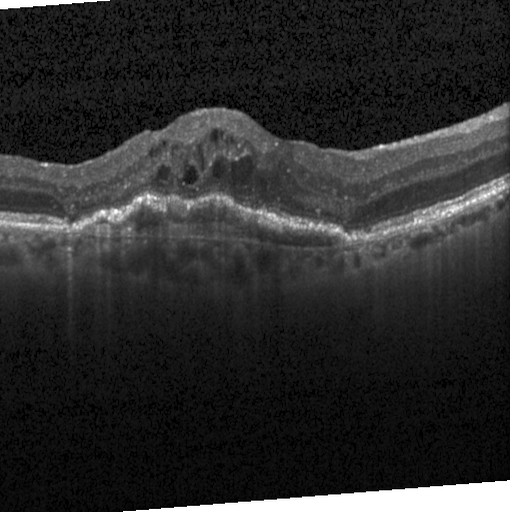

Optical coherence tomography scan. Horizontal scan through the fovea
Impression: DME.